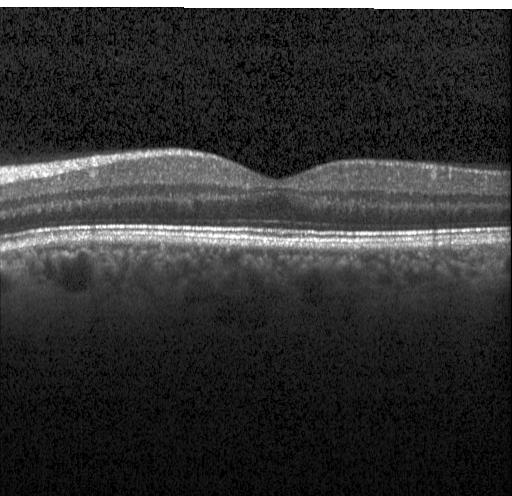
Through the macula · spectral-domain OCT · Heidelberg Spectralis OCT system · optical coherence tomography B-scan. This B-scan demonstrates no evidence of choroidal neovascularization, diabetic macular edema, or drusen.